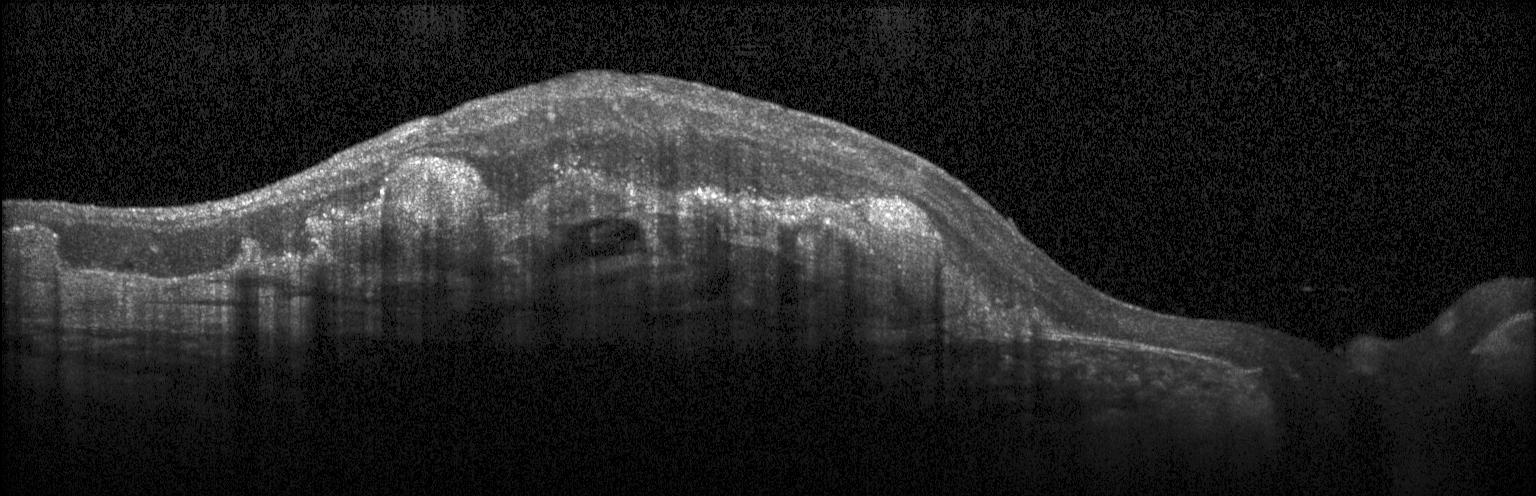 Retinal OCT B-scan
Assessment: a choroidal neovascular membrane.